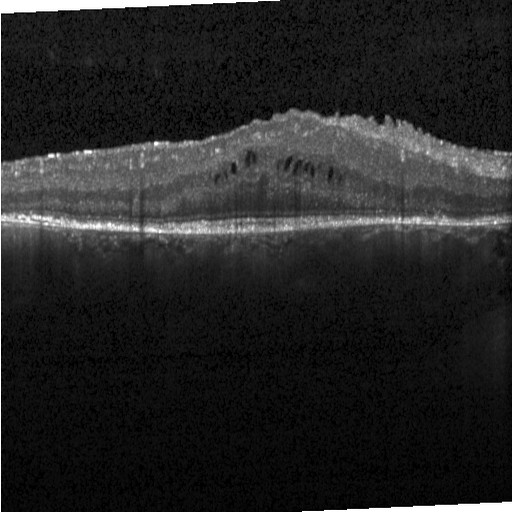
Horizontal scan through the fovea; instrument: Heidelberg Spectralis; OCT line scan.
This B-scan demonstrates diabetic macular edema (DME).